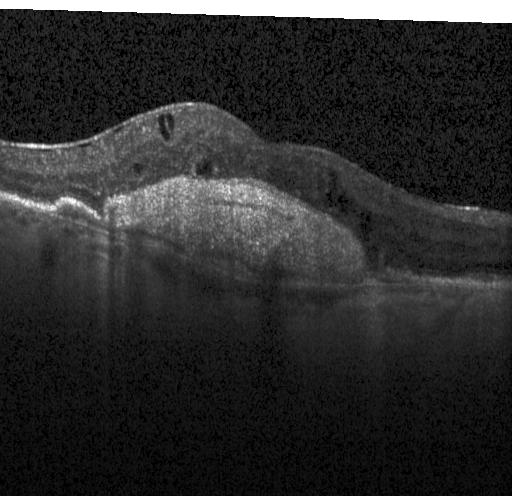

Macular scan, retinal OCT B-scan — Assessment: choroidal neovascularization.